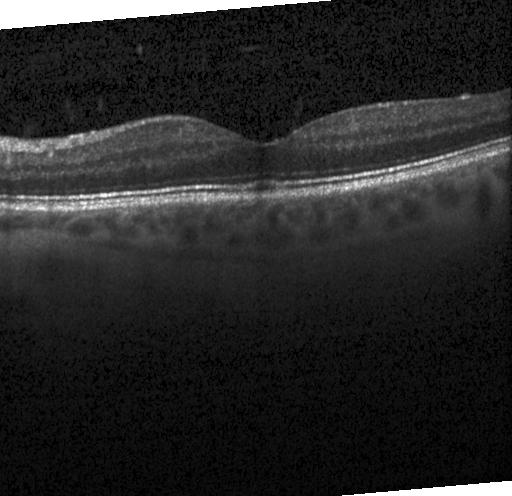
OCT B-scan, Heidelberg Spectralis
Diagnosis: neither choroidal neovascularization, diabetic macular edema, nor drusen.